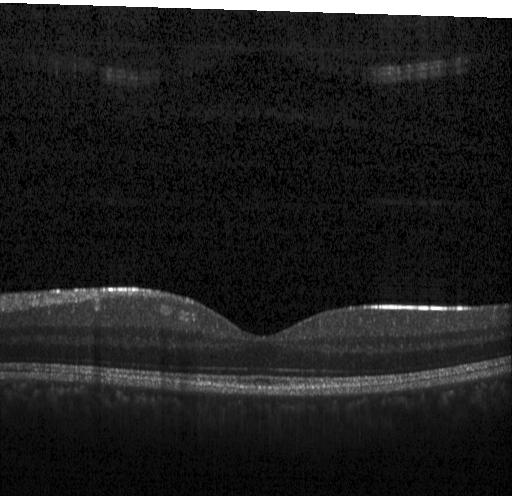 Spectral-domain OCT B-scan: neither choroidal neovascularization, diabetic macular edema, nor drusen.